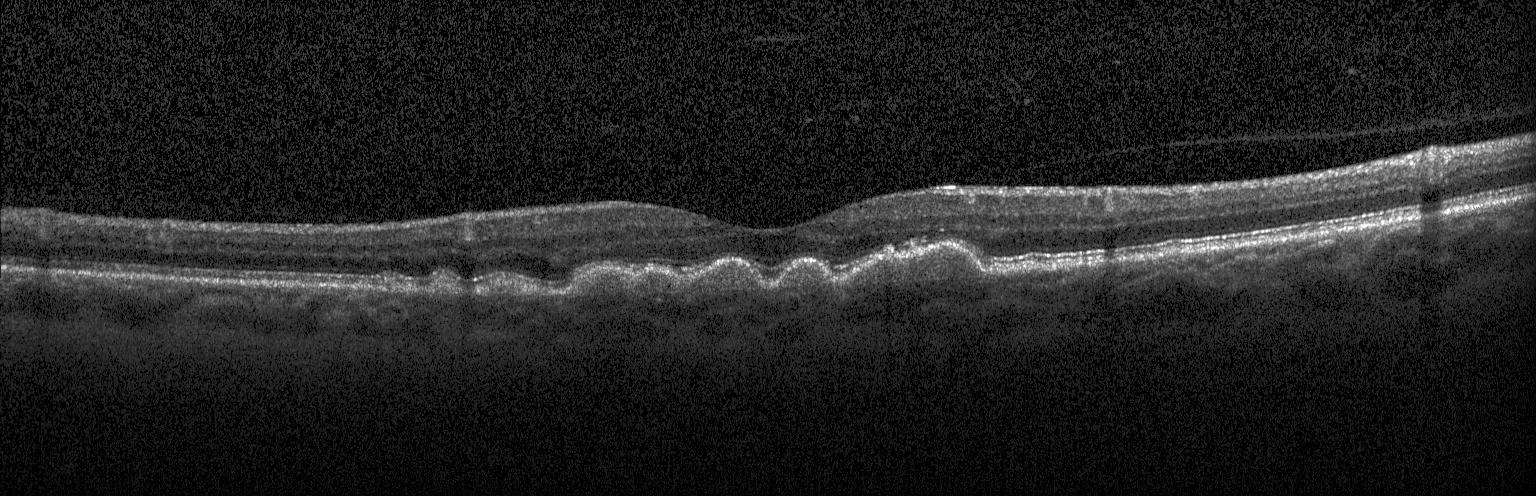
OCT B-scan — Impression: multiple drusen.